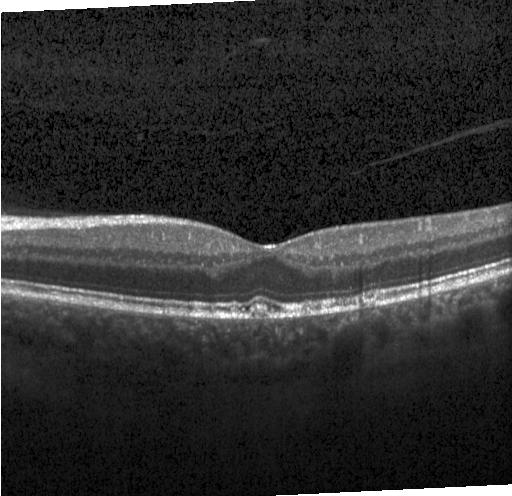 SD-OCT · Heidelberg Spectralis OCT system · centered on the fovea · optical coherence tomography B-scan.
Impression: drusen.